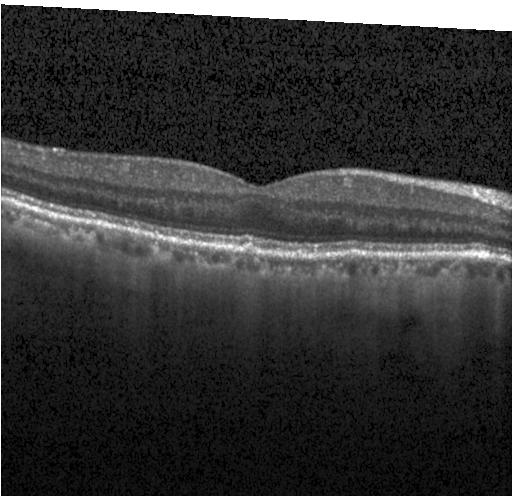 Horizontal scan through the fovea · optical coherence tomography scan · spectral-domain OCT · instrument: Heidelberg Spectralis. Multiple drusen.